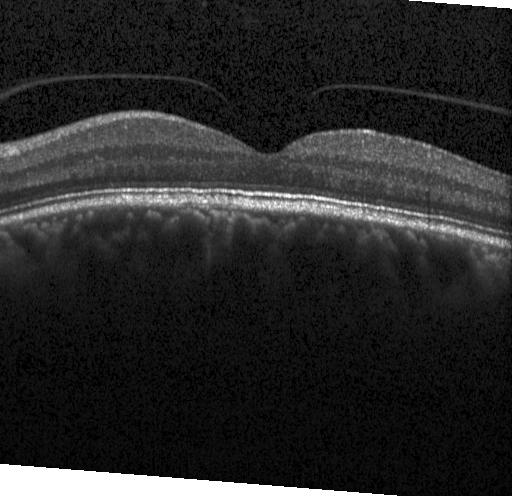 Dx: neither choroidal neovascularization, diabetic macular edema, nor drusen.